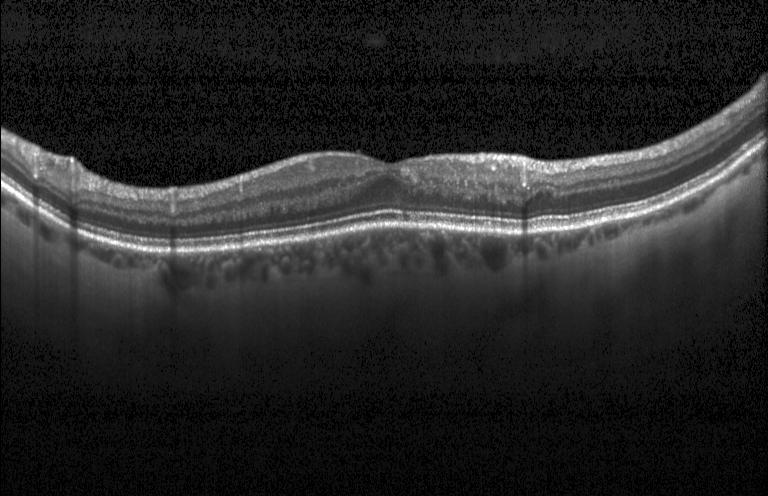
SD-OCT; retinal OCT cross-section; macular scan — Impression: neither choroidal neovascularization, diabetic macular edema, nor drusen.